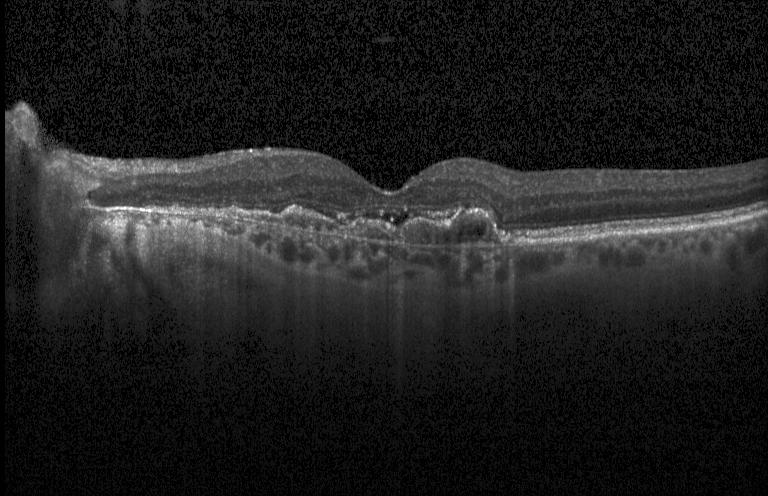
Fovea-centered. Retinal OCT cross-section. Spectral-domain optical coherence tomography — OCT finding: a choroidal neovascular membrane.